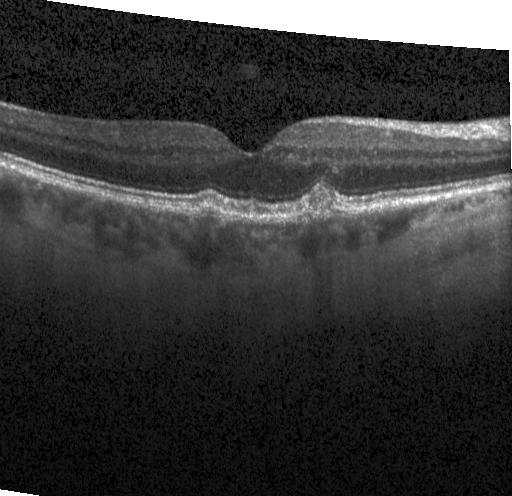

OCT finding: multiple drusen.